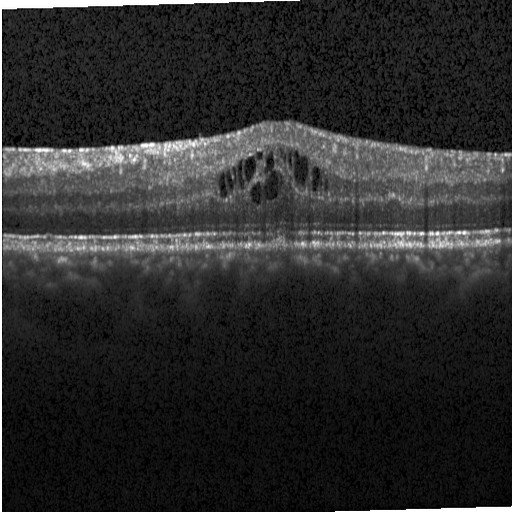

SD-OCT, through the macula, optical coherence tomography B-scan.
DME.